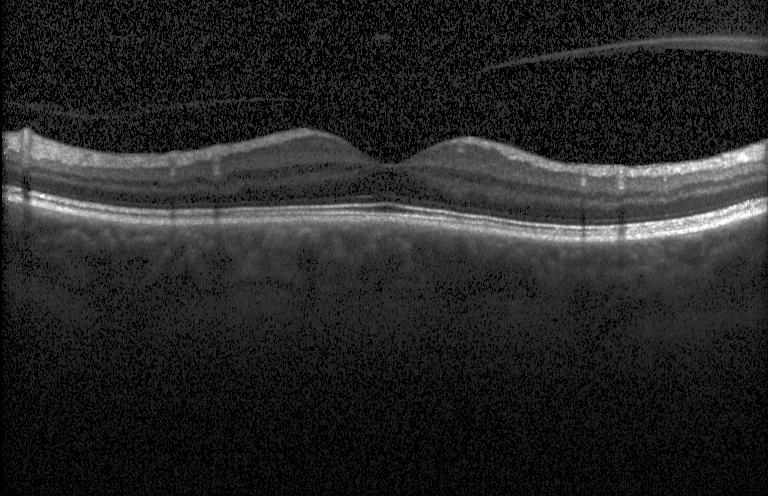

Spectral-domain OCT. Horizontal scan through the fovea. Optical coherence tomography scan.
Neither CNV, DME, nor drusen.